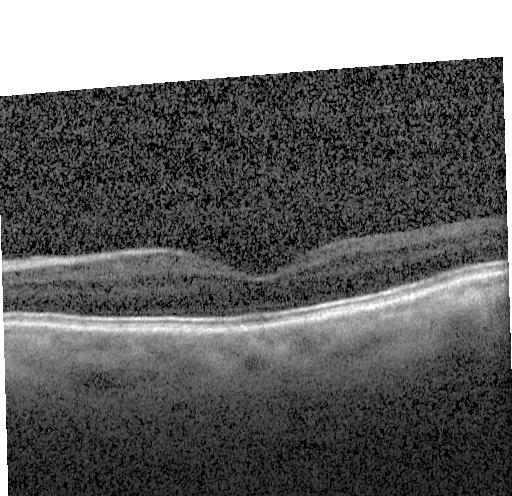 Dx: no evidence of choroidal neovascularization, diabetic macular edema, or drusen.